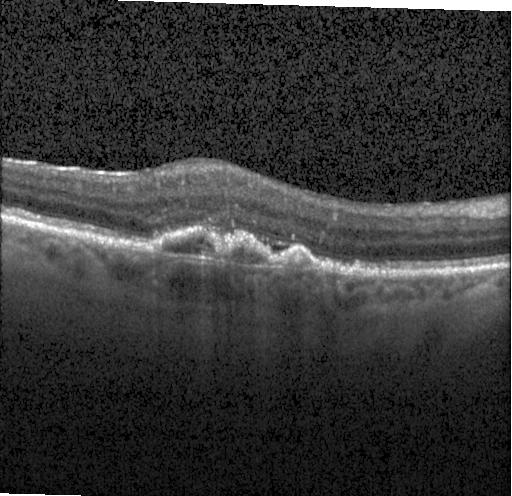 Heidelberg Spectralis · OCT B-scan · SD-OCT · fovea-centered — Finding: a choroidal neovascular membrane.